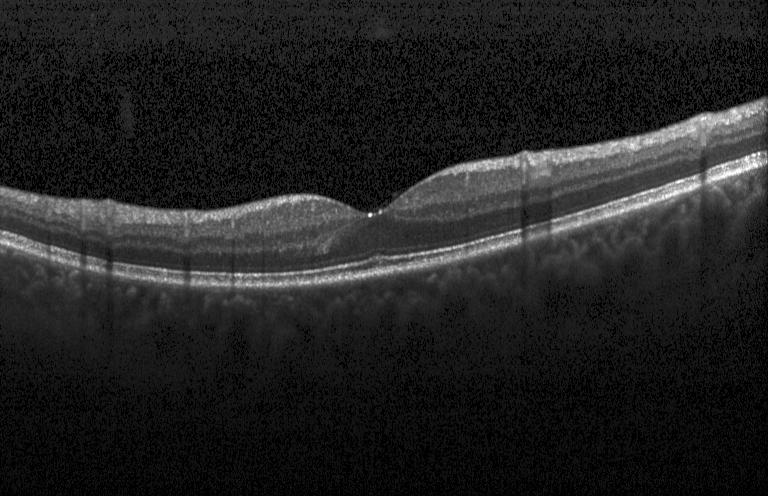
Spectral-domain OCT. Horizontal scan through the fovea. Optical coherence tomography B-scan. Instrument: Heidelberg Spectralis. Dx: no choroidal neovascularization, diabetic macular edema, or drusen.